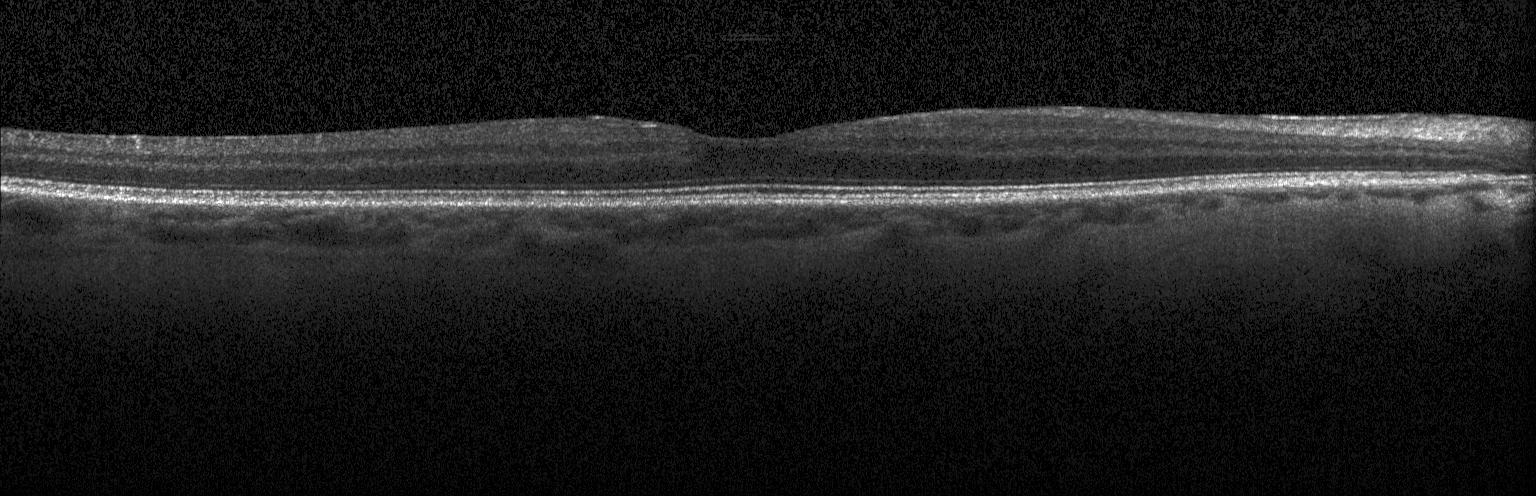
Retinal OCT B-scan
This B-scan demonstrates no evidence of choroidal neovascularization, diabetic macular edema, or drusen.